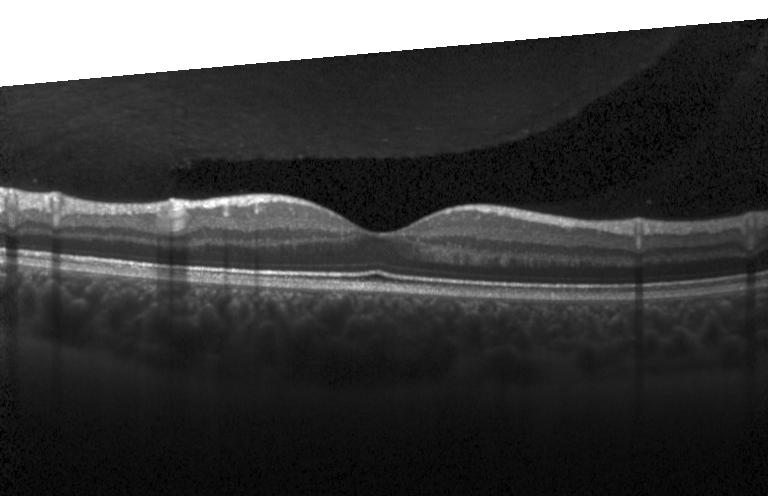
Dx: no choroidal neovascularization, no diabetic macular edema, and no drusen.